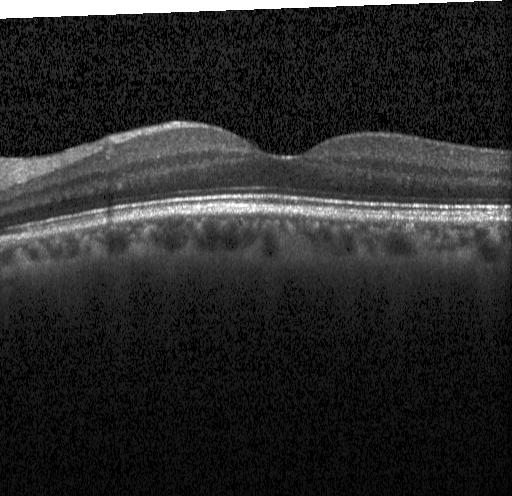
Finding: no choroidal neovascularization, diabetic macular edema, or drusen.